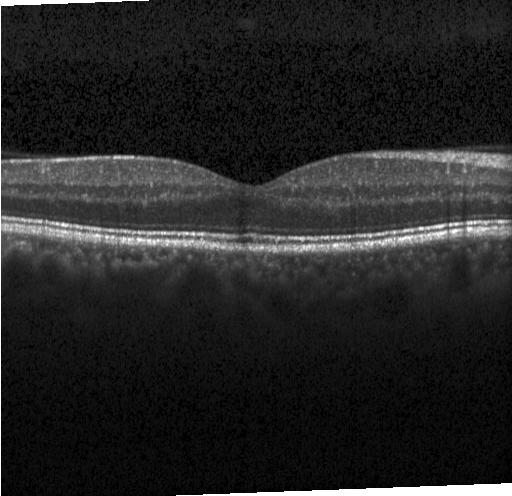 Finding: no choroidal neovascularization, diabetic macular edema, or drusen.